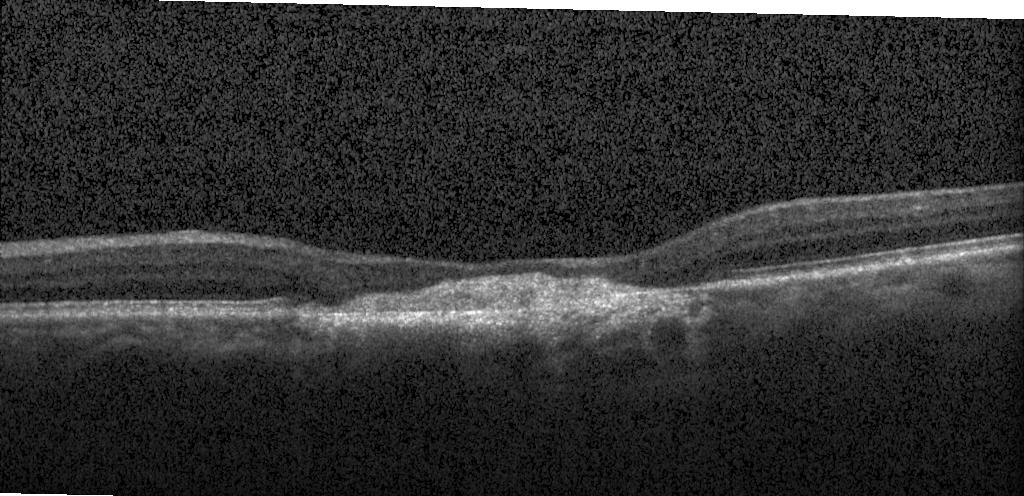

Optical coherence tomography scan, spectral-domain optical coherence tomography, Heidelberg Spectralis, through the macula — This B-scan demonstrates a choroidal neovascular membrane.